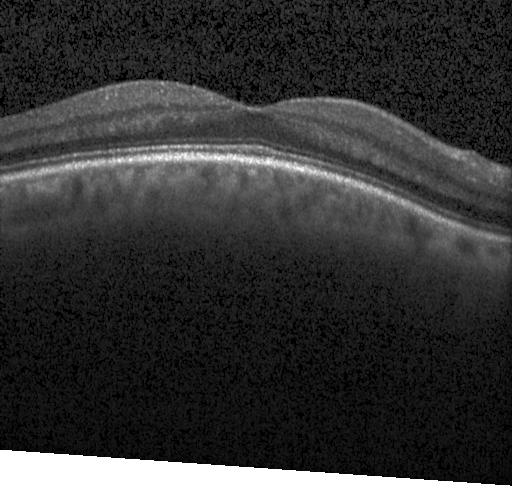
Heidelberg Spectralis, SD-OCT, horizontal scan through the fovea, retinal OCT cross-section. Finding: no evidence of choroidal neovascularization, diabetic macular edema, or drusen.